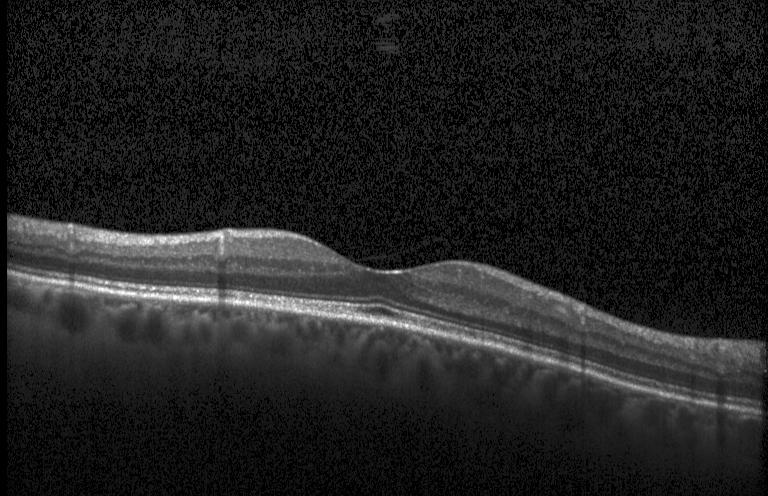
OCT B-scan; spectral-domain optical coherence tomography — Diagnosis: no CNV, no DME, and no drusen.